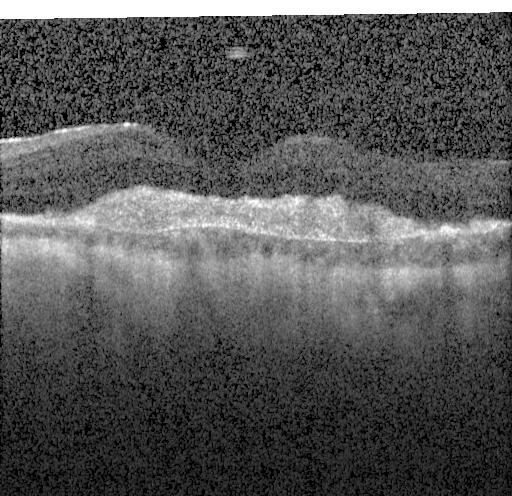 Impression: a choroidal neovascular membrane.